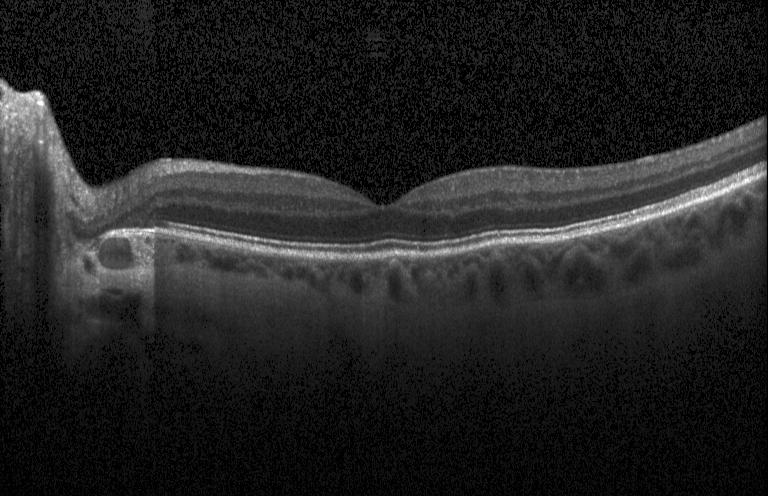 Fovea-centered, retinal OCT cross-section, Heidelberg Spectralis.
Macular OCT: no CNV, DME, or drusen.